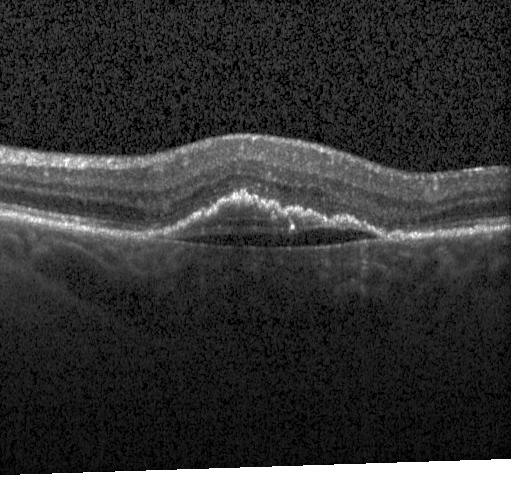 Spectral-domain OCT B-scan: choroidal neovascularization.